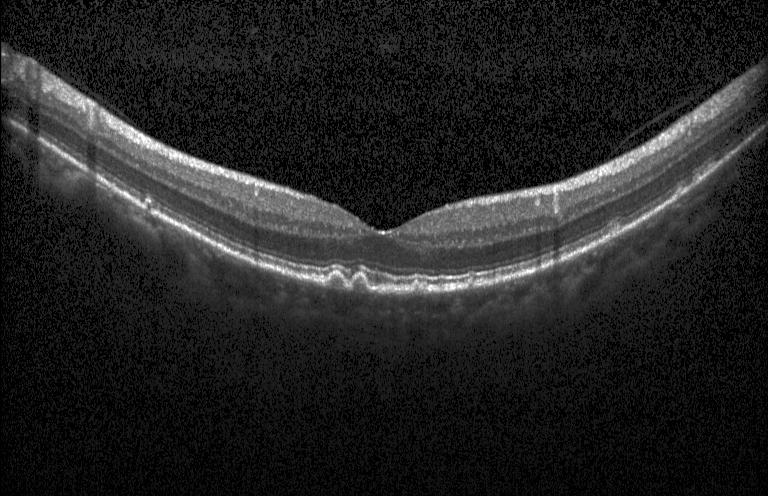
Instrument: Heidelberg Spectralis · optical coherence tomography scan — Drusen.